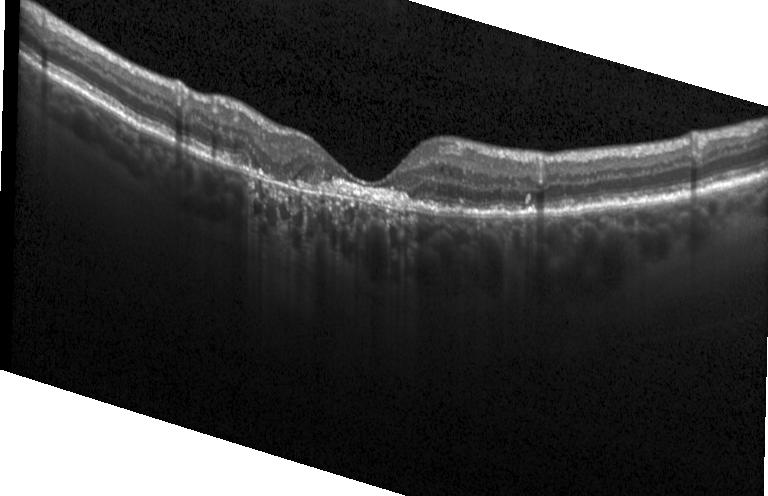

Diagnosis: a choroidal neovascular membrane.